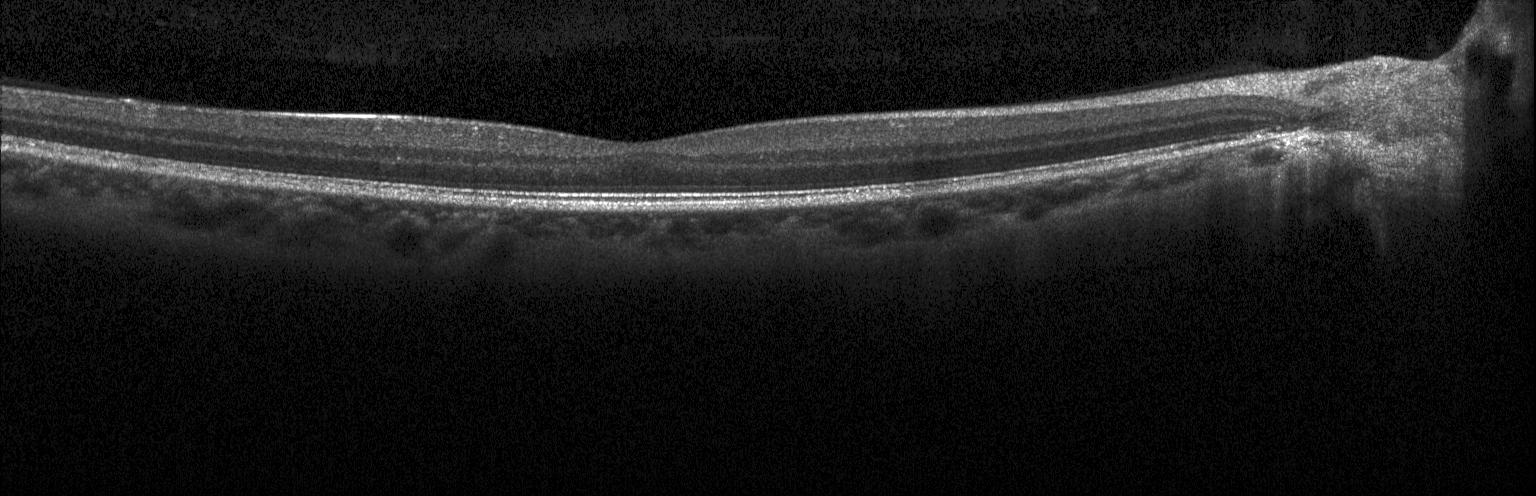

Impression: no choroidal neovascularization, no diabetic macular edema, and no drusen.